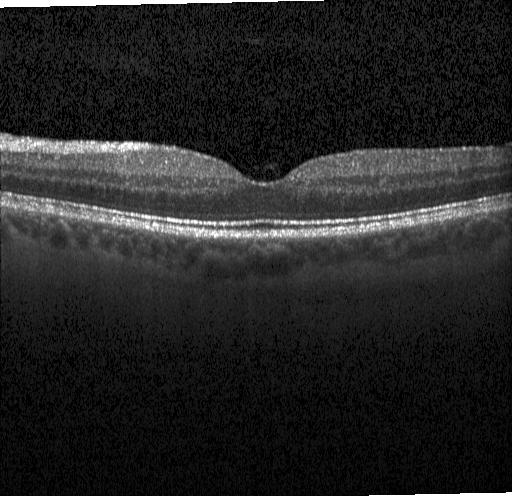 This B-scan demonstrates no evidence of CNV, DME, or drusen.